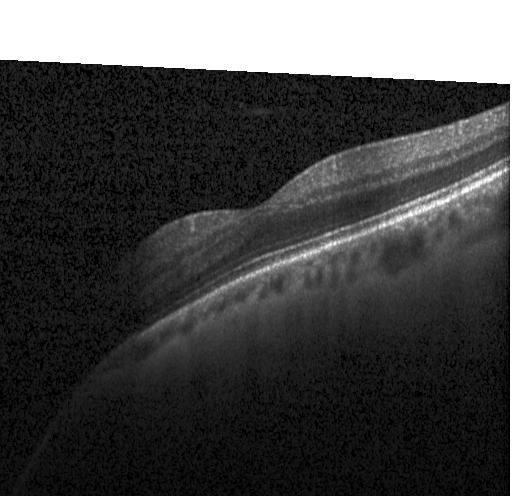

Heidelberg Spectralis OCT system, optical coherence tomography B-scan.
Impression: no choroidal neovascularization, no diabetic macular edema, and no drusen.